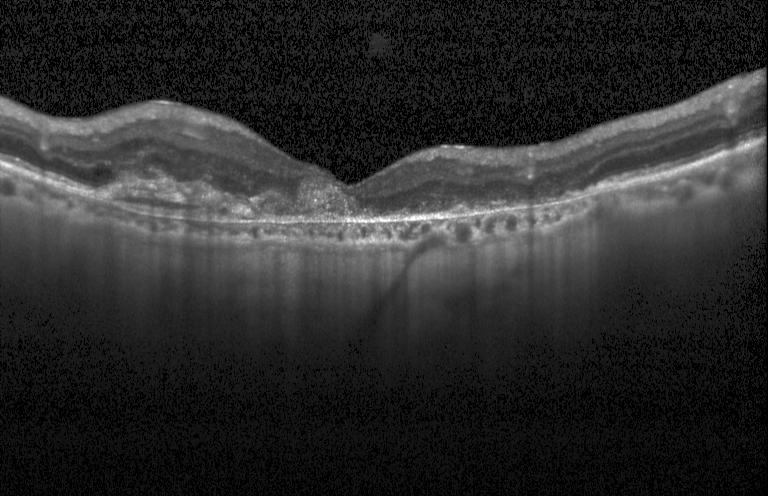
Finding: a choroidal neovascular membrane.